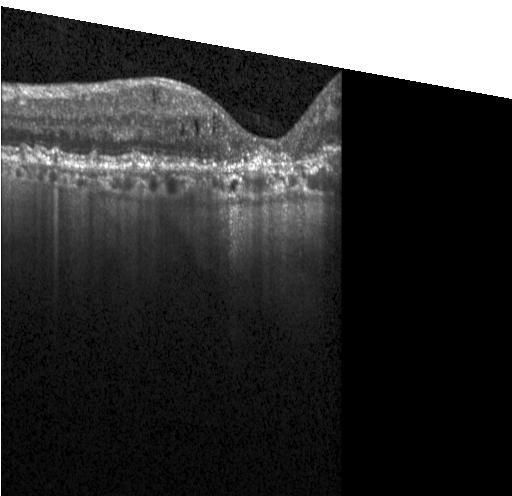

Macular OCT demonstrating a choroidal neovascular membrane.